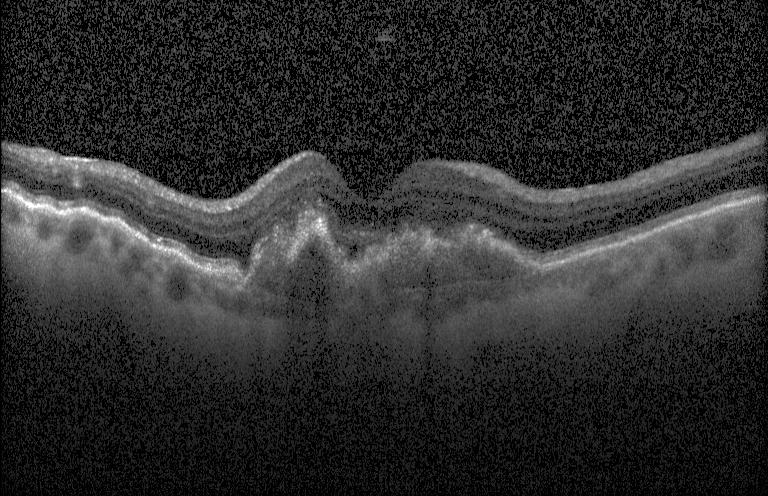
Heidelberg Spectralis OCT system. Retinal OCT cross-section. Impression: choroidal neovascularization (CNV).